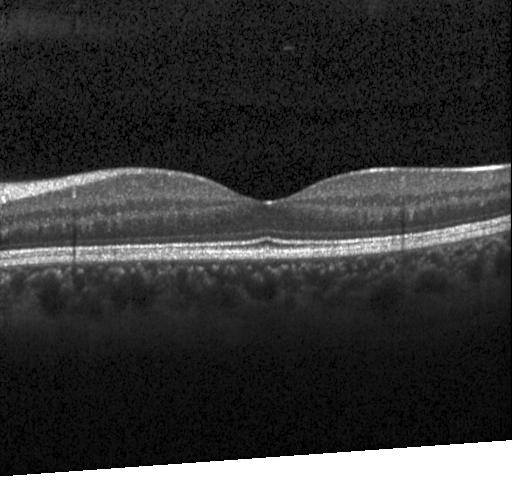 Heidelberg Spectralis · through the macula · OCT line scan · spectral-domain OCT.
Diagnosis: no choroidal neovascularization, diabetic macular edema, or drusen.